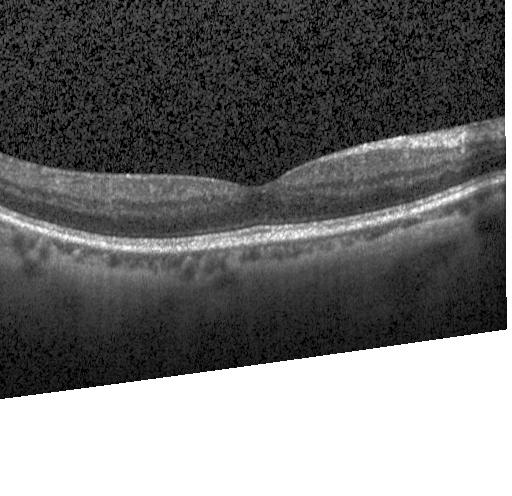
Spectral-domain OCT B-scan: neither CNV, DME, nor drusen.